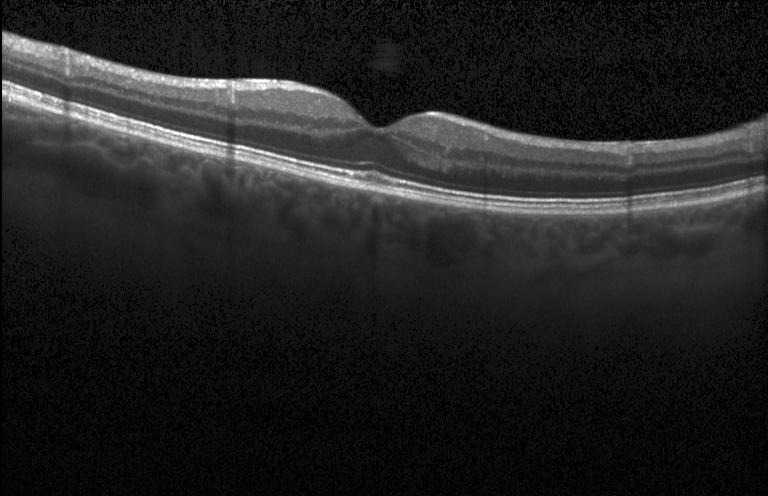

Assessment: no evidence of choroidal neovascularization, diabetic macular edema, or drusen.